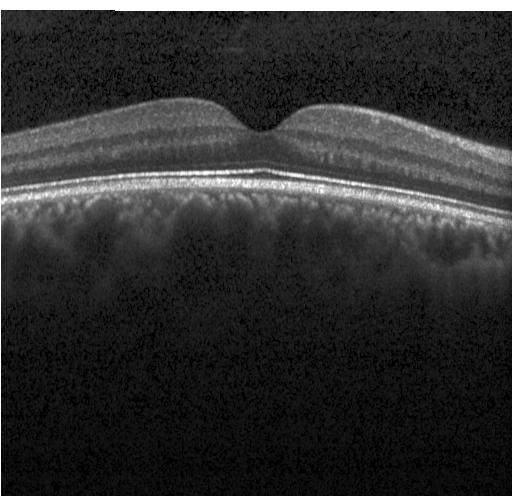
SD-OCT; optical coherence tomography scan
Assessment: no choroidal neovascularization, no diabetic macular edema, and no drusen.